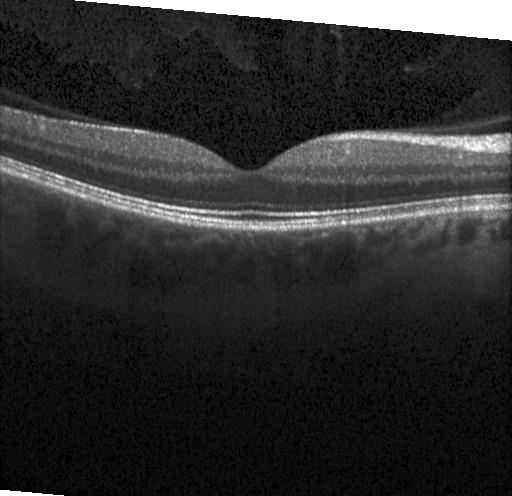
Spectral-domain optical coherence tomography, instrument: Heidelberg Spectralis, optical coherence tomography scan. Assessment: no evidence of choroidal neovascularization, diabetic macular edema, or drusen.